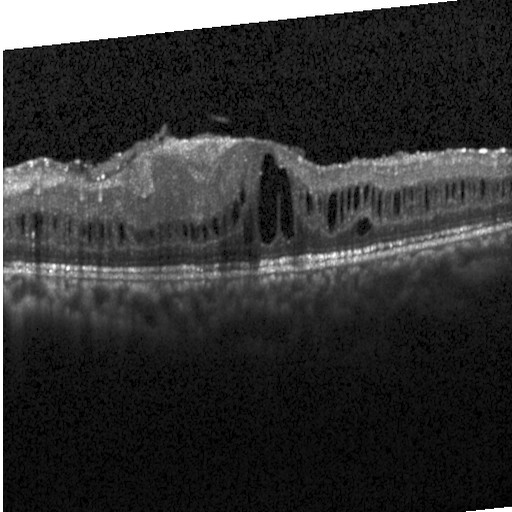

DME.